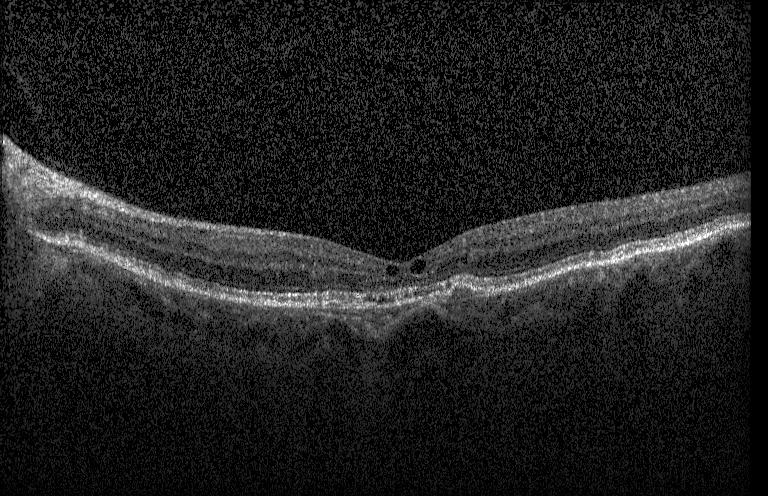
Retinal OCT B-scan; spectral-domain optical coherence tomography; Heidelberg Spectralis — Finding: a choroidal neovascular membrane.